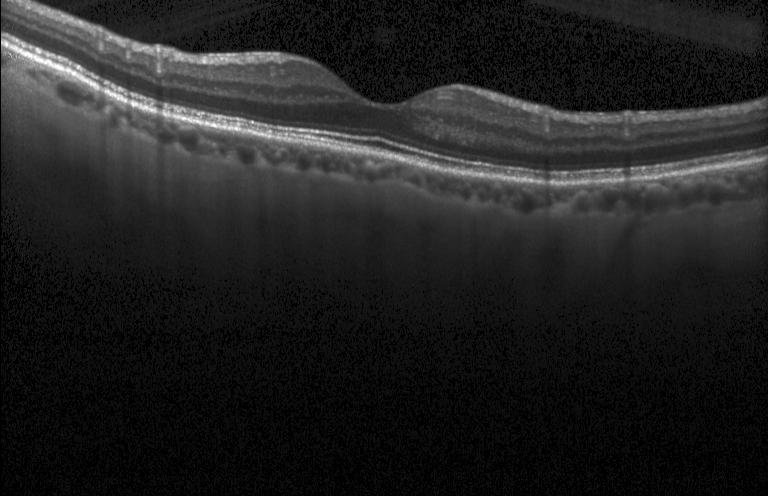

Optical coherence tomography scan — OCT finding: no evidence of CNV, DME, or drusen.